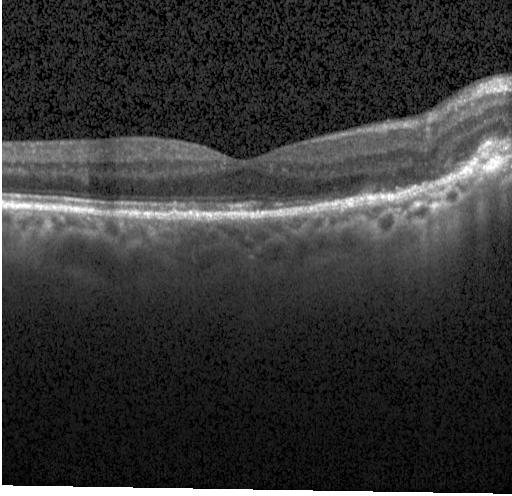 Fovea-centered, instrument: Heidelberg Spectralis, OCT line scan, spectral-domain optical coherence tomography
Impression: a choroidal neovascular membrane.